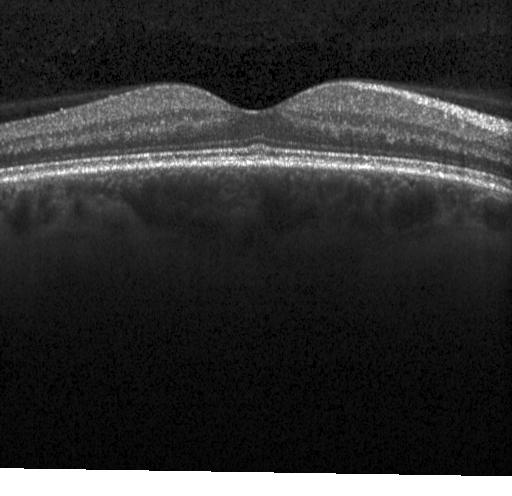 Spectral-domain OCT · retinal OCT B-scan · macular scan · Heidelberg Spectralis
The scan shows no evidence of choroidal neovascularization, diabetic macular edema, or drusen.